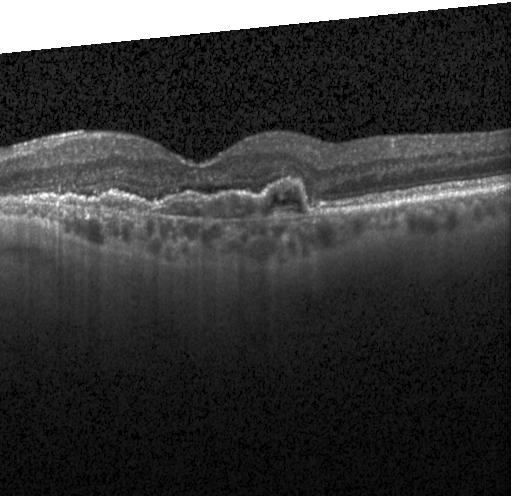
Finding: CNV.